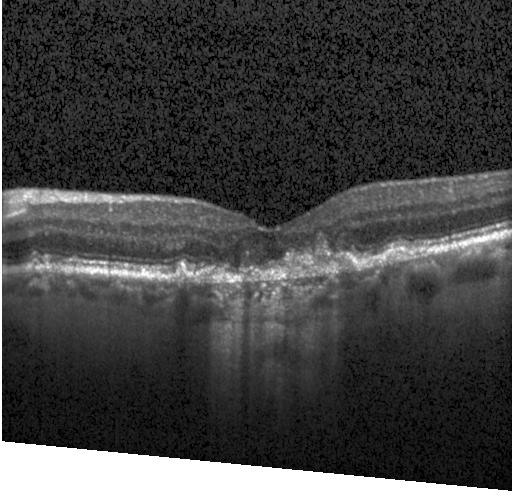 A choroidal neovascular membrane.